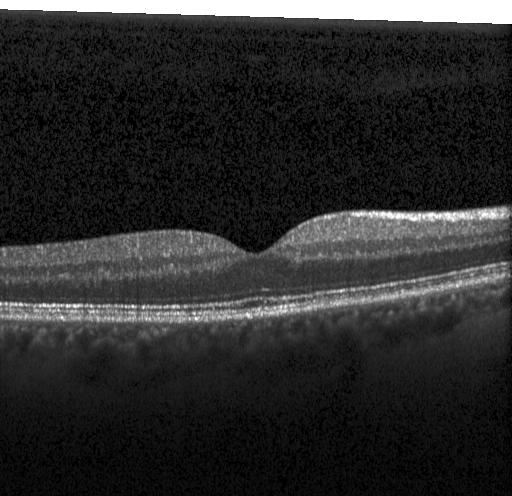

Impression: neither choroidal neovascularization, diabetic macular edema, nor drusen.